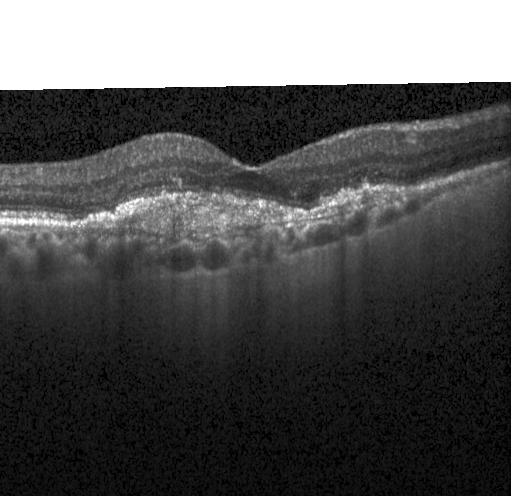
Acquired on a Heidelberg Spectralis; centered on the fovea; OCT B-scan; spectral-domain optical coherence tomography. The scan shows a choroidal neovascular membrane.